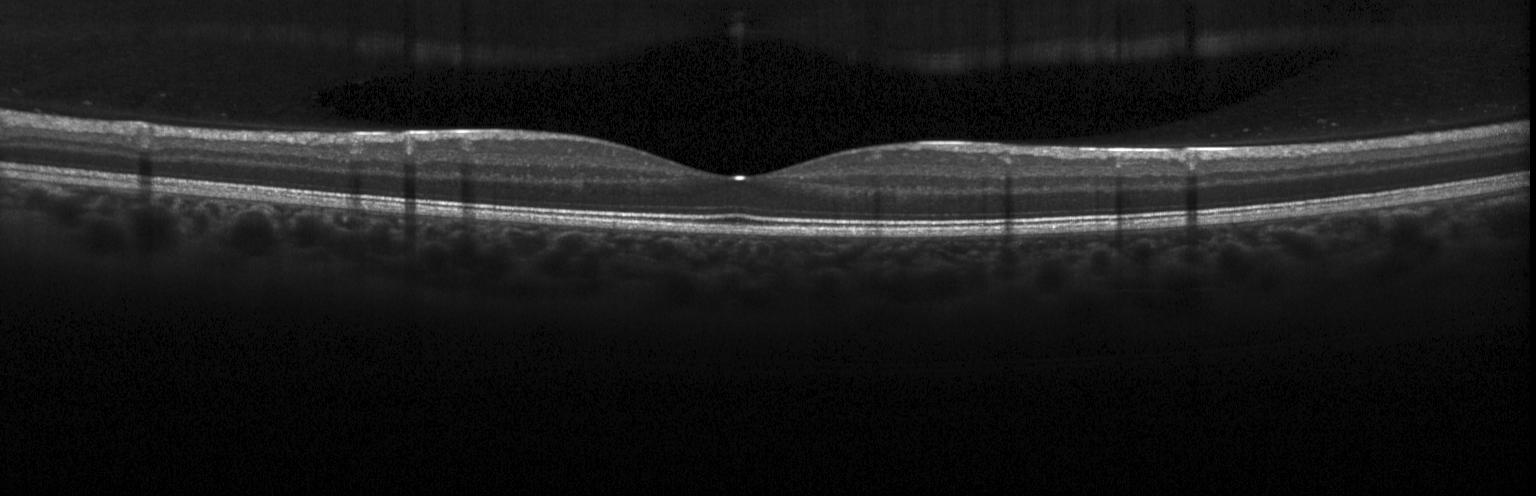 Spectral-domain OCT · retinal OCT cross-section.
No evidence of choroidal neovascularization, diabetic macular edema, or drusen.